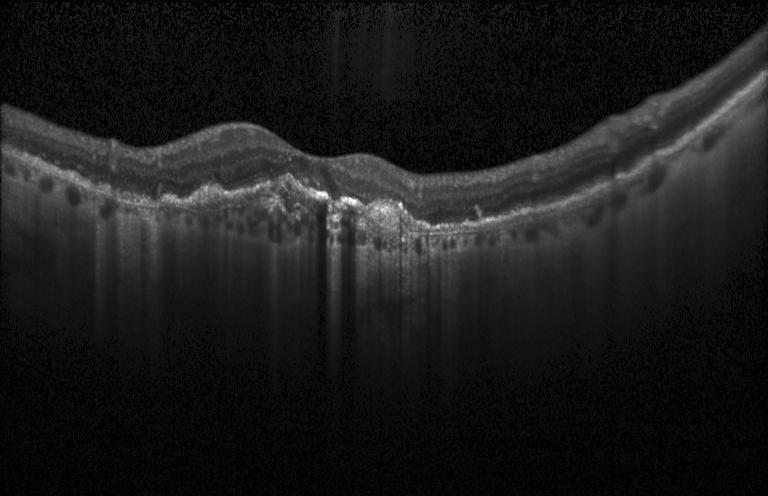

OCT B-scan · SD-OCT
Impression: a choroidal neovascular membrane.